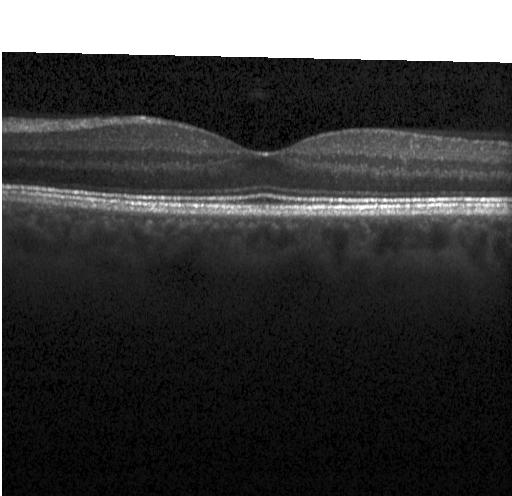
Retinal OCT cross-section; Heidelberg Spectralis OCT system; centered on the fovea — The scan shows neither choroidal neovascularization, diabetic macular edema, nor drusen.